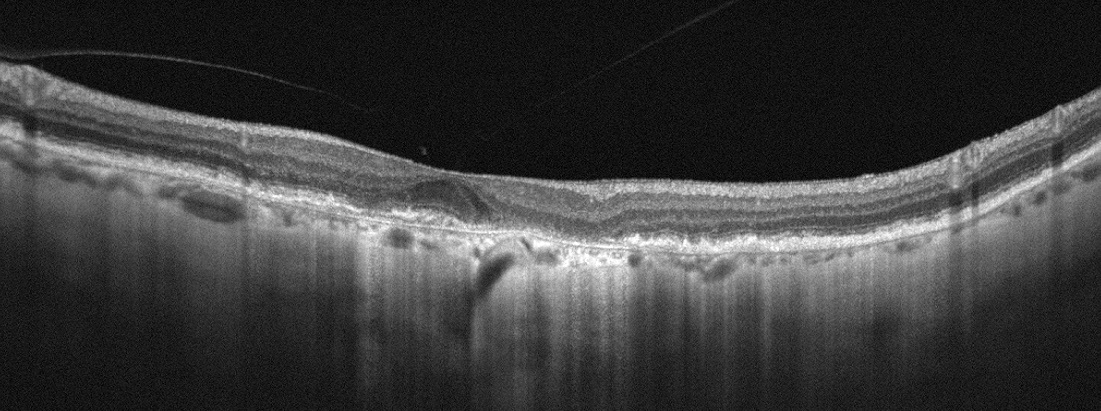

Optovue Avanti RTVue XR. Retinal OCT cross-section. Through the macula. The scan shows age-related macular degeneration (AMD).